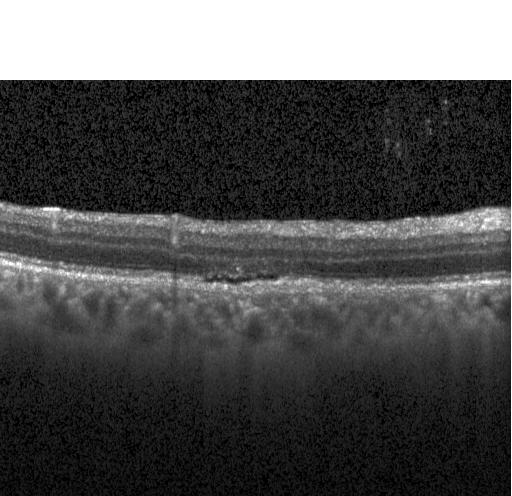 The scan shows choroidal neovascularization (CNV).